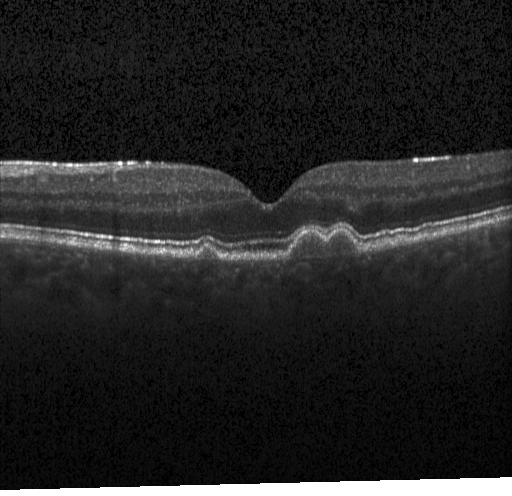 Retinal OCT cross-section showing drusen.